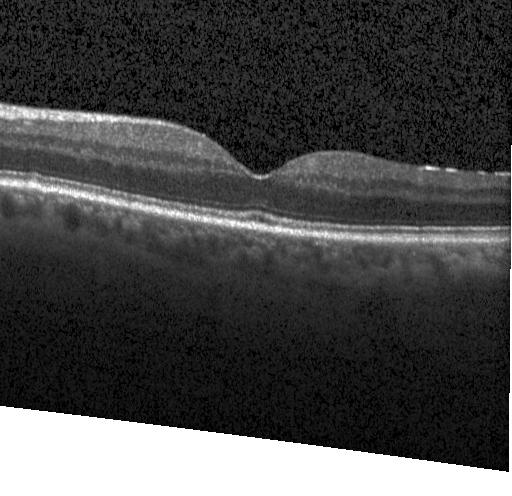
Retinal OCT cross-section showing no evidence of CNV, DME, or drusen.